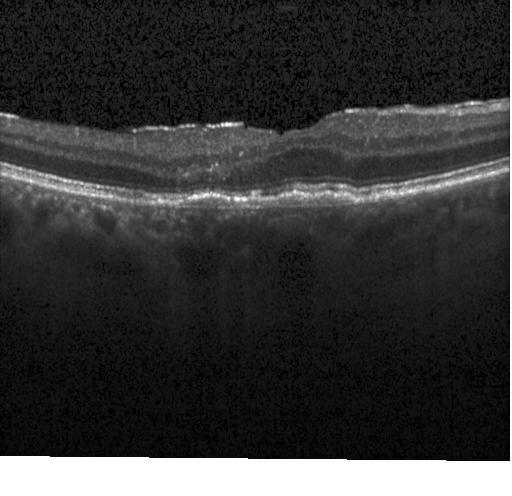
Spectral-domain optical coherence tomography; retinal OCT cross-section; Heidelberg Spectralis; through the macula — Assessment: a choroidal neovascular membrane.